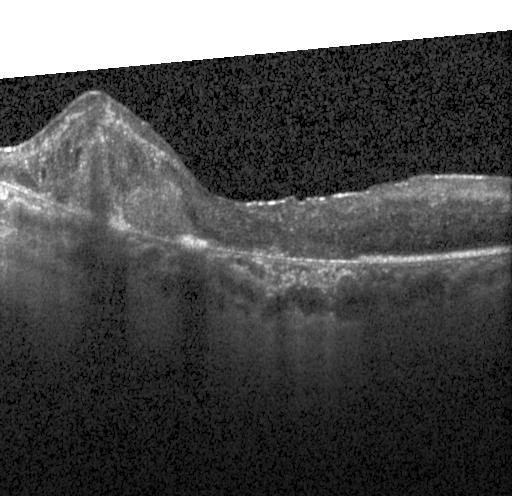 This B-scan demonstrates CNV.